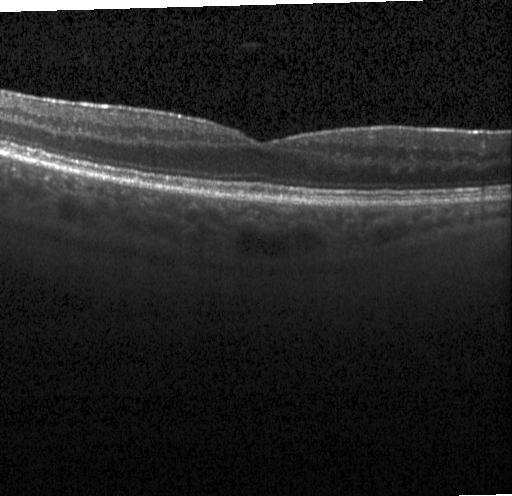
Dx: no choroidal neovascularization, no diabetic macular edema, and no drusen.